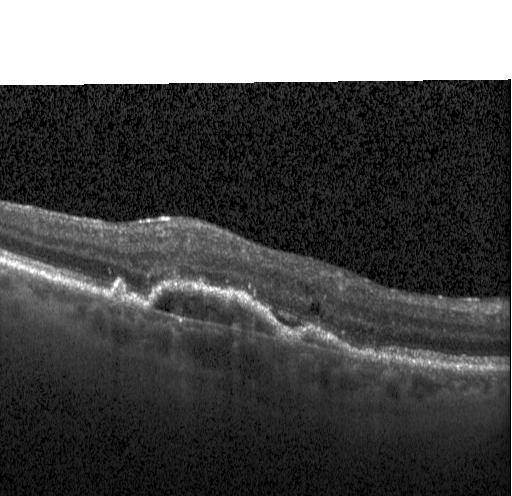

Macular OCT: a choroidal neovascular membrane.